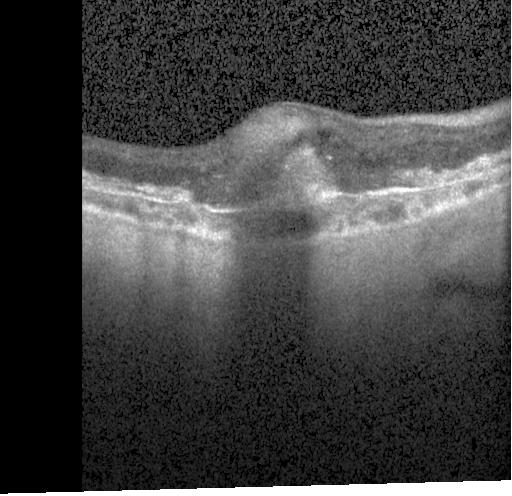
Finding: a choroidal neovascular membrane.